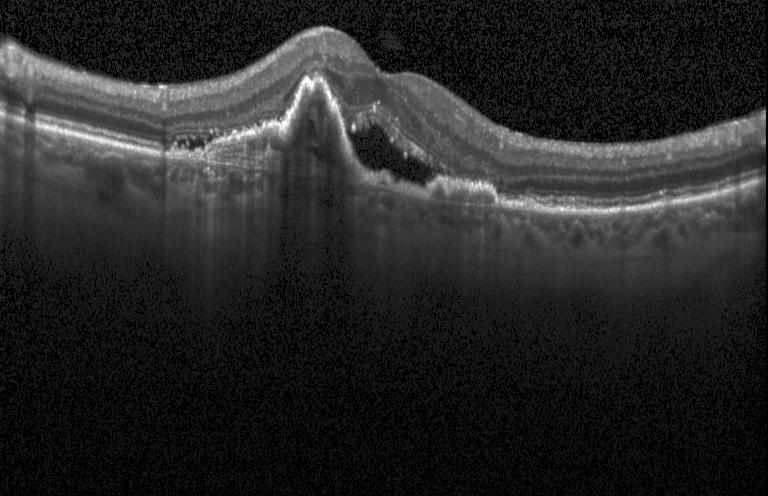

Spectral-domain OCT · retinal OCT B-scan · Heidelberg Spectralis OCT system
Macular OCT: a choroidal neovascular membrane.